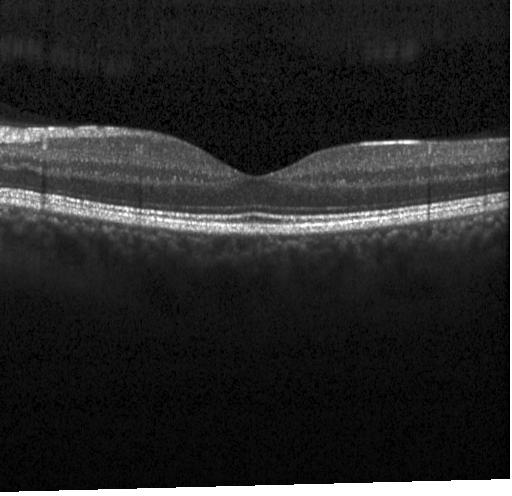 Macular OCT demonstrating neither choroidal neovascularization, diabetic macular edema, nor drusen.